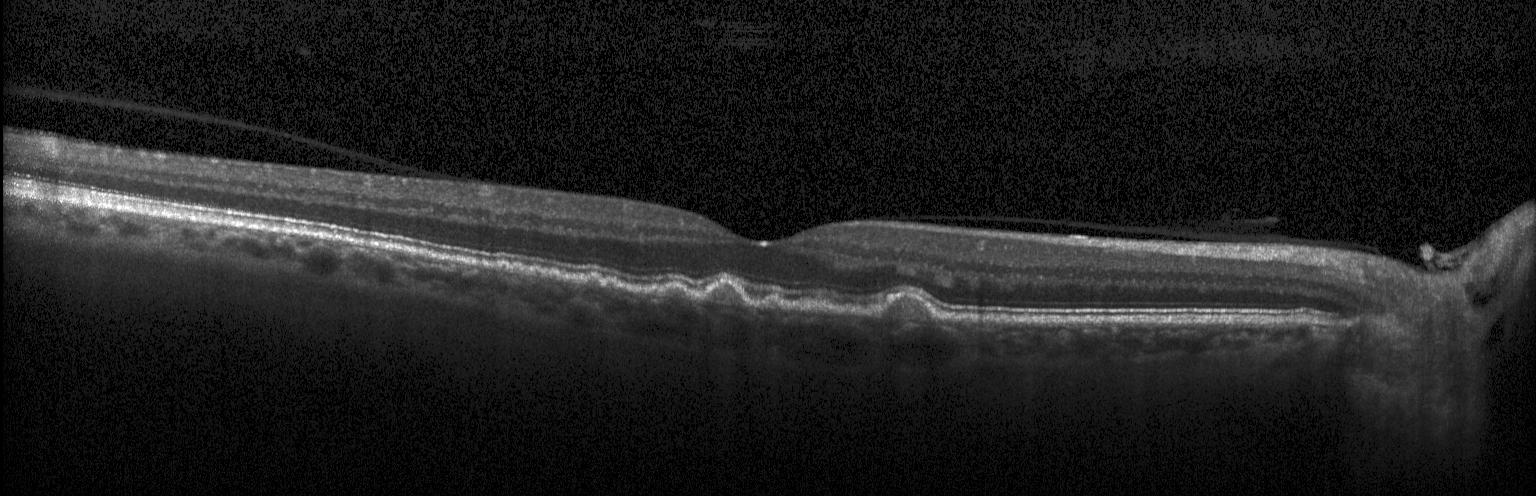 Dx: drusen.